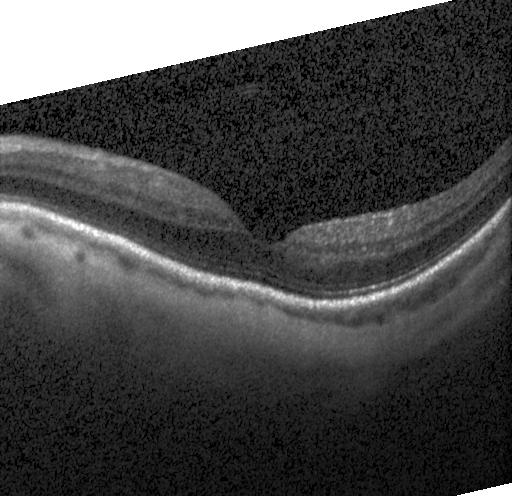

Optical coherence tomography B-scan — Finding: no CNV, DME, or drusen.